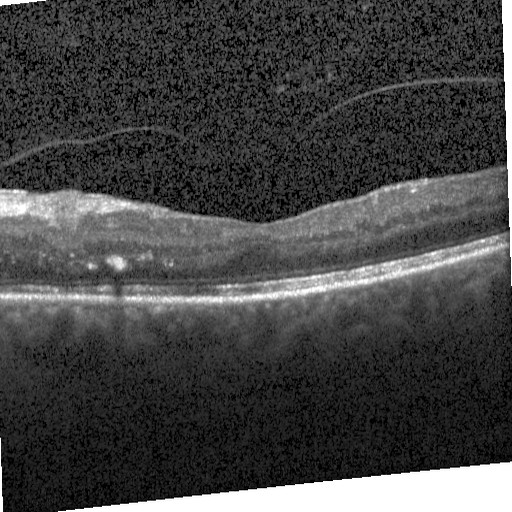
OCT finding: diabetic macular edema.